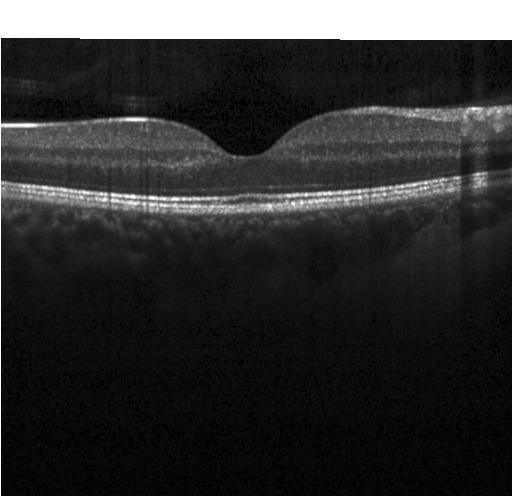 OCT B-scan, instrument: Heidelberg Spectralis. Finding: no CNV, no DME, and no drusen.